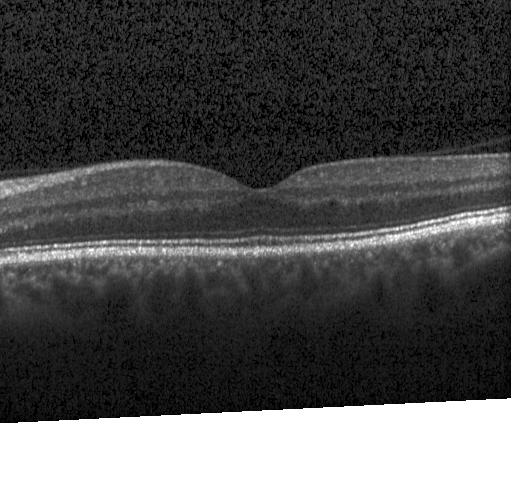 OCT B-scan. Spectral-domain OCT.
Finding: neither choroidal neovascularization, diabetic macular edema, nor drusen.